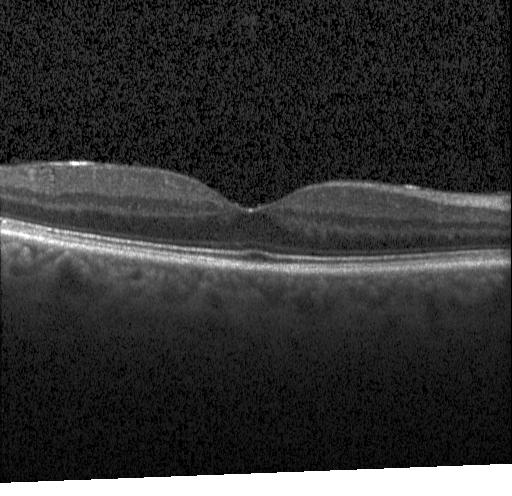 Retinal OCT cross-section · macular scan · instrument: Heidelberg Spectralis · SD-OCT
This B-scan demonstrates no choroidal neovascularization, diabetic macular edema, or drusen.